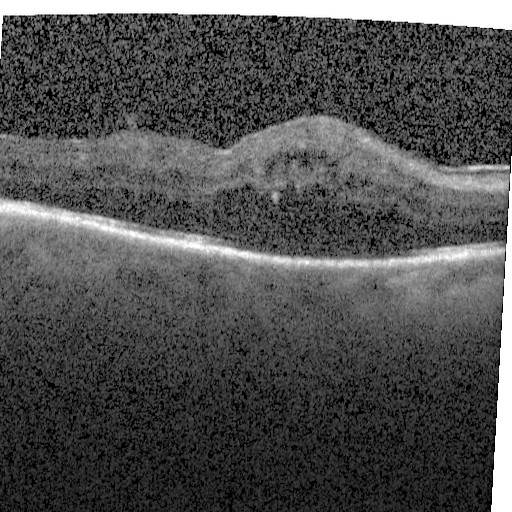 Heidelberg Spectralis · horizontal scan through the fovea · optical coherence tomography scan · spectral-domain OCT. Diagnosis: DME.